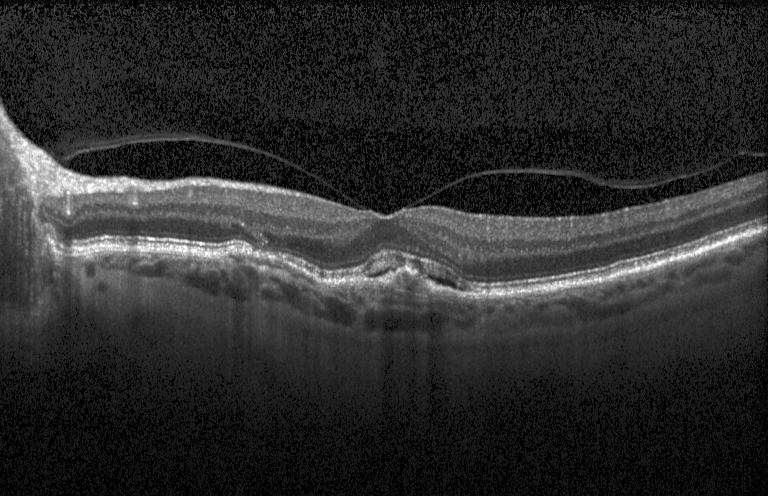

Retinal OCT cross-section · acquired on a Heidelberg Spectralis · SD-OCT · centered on the fovea. A choroidal neovascular membrane.